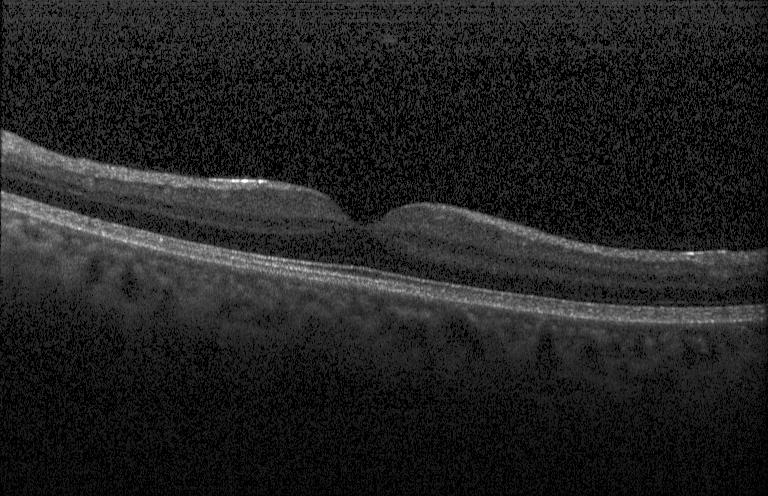

Optical coherence tomography B-scan. Macular OCT: no choroidal neovascularization, diabetic macular edema, or drusen.